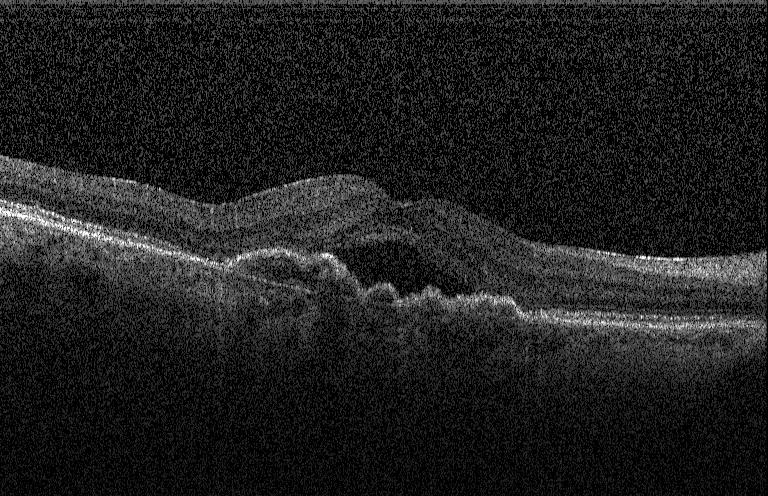

Retinal OCT cross-section — The scan shows a choroidal neovascular membrane.